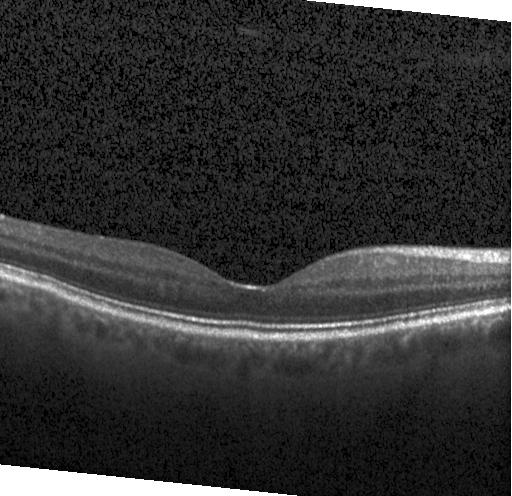

Impression: neither choroidal neovascularization, diabetic macular edema, nor drusen.